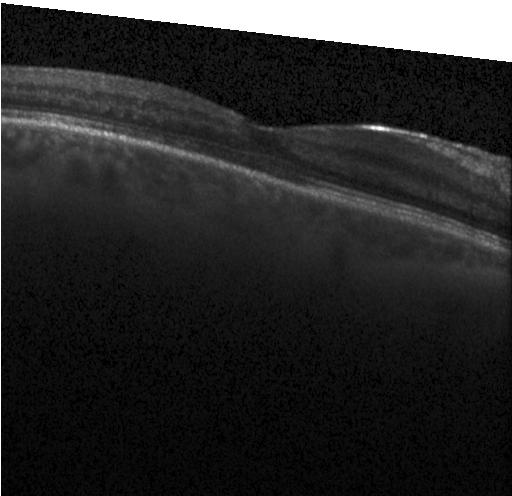

Macular scan; instrument: Heidelberg Spectralis; retinal OCT cross-section.
Diagnosis: no choroidal neovascularization, no diabetic macular edema, and no drusen.